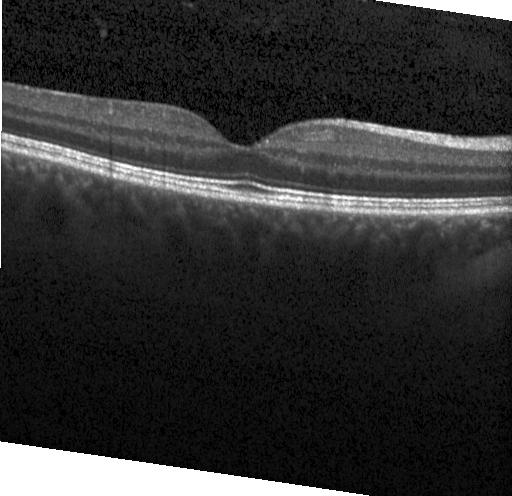
Optical coherence tomography scan
OCT finding: no choroidal neovascularization, diabetic macular edema, or drusen.